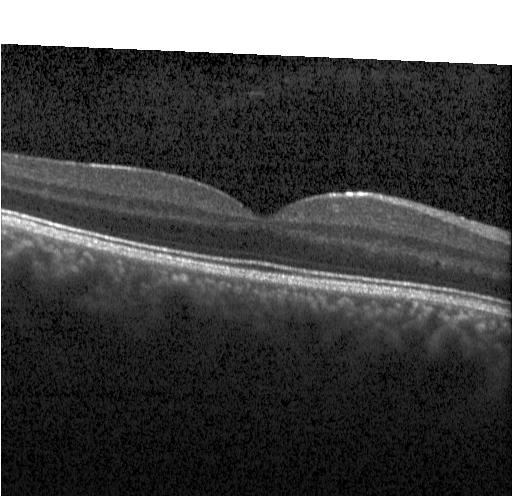
OCT line scan, spectral-domain OCT, Heidelberg Spectralis OCT system.
Assessment: no choroidal neovascularization, diabetic macular edema, or drusen.